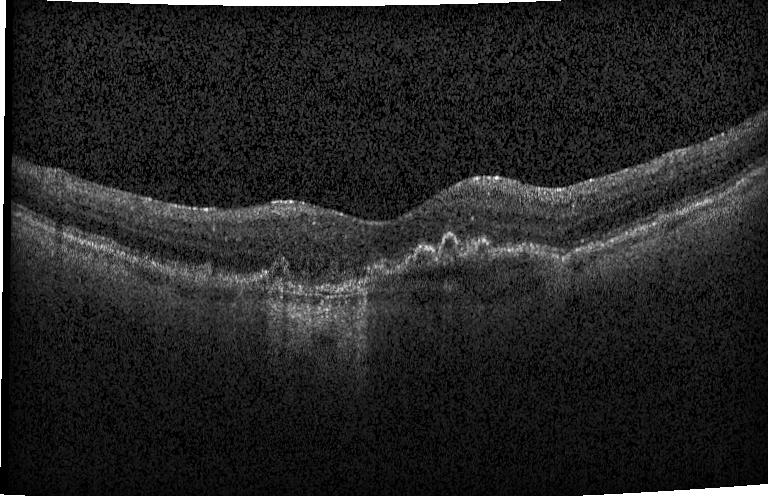

Dx: choroidal neovascularization (CNV).